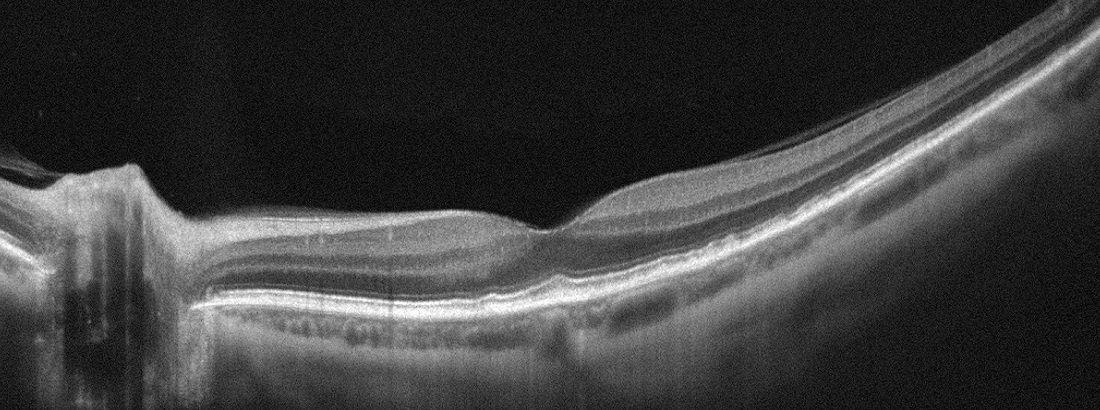 Retinal OCT cross-section. Optovue Avanti RTVue XR. Fovea-centered — Finding: age-related macular degeneration (AMD).